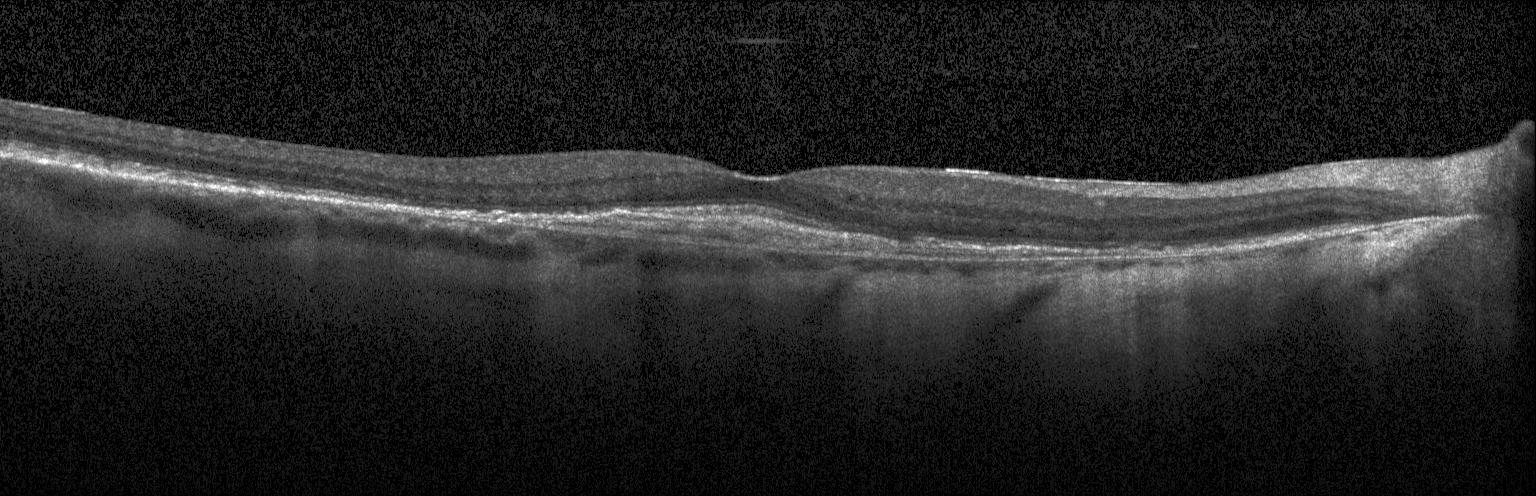

OCT B-scan showing CNV.